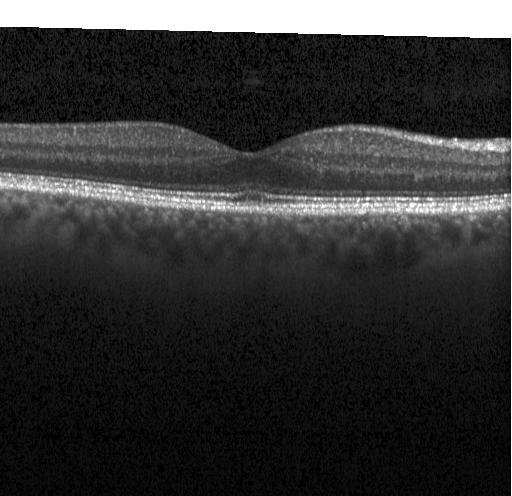
Spectral-domain OCT B-scan: no evidence of choroidal neovascularization, diabetic macular edema, or drusen.